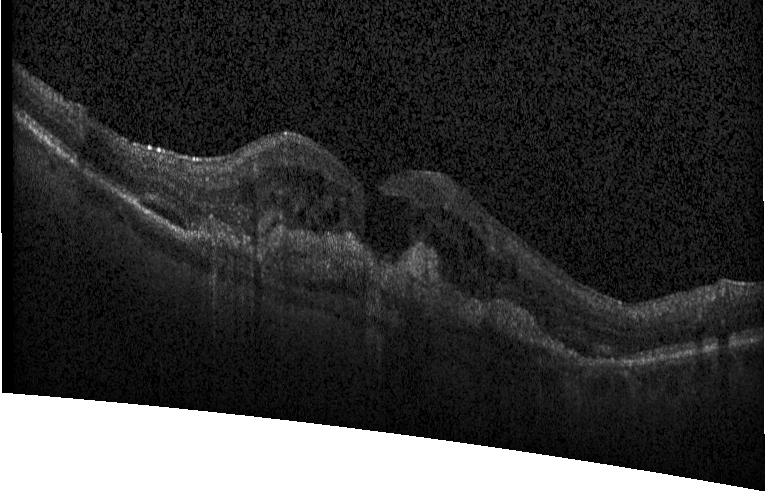

Spectral-domain optical coherence tomography; Heidelberg Spectralis OCT system; fovea-centered; OCT line scan
Impression: CNV.